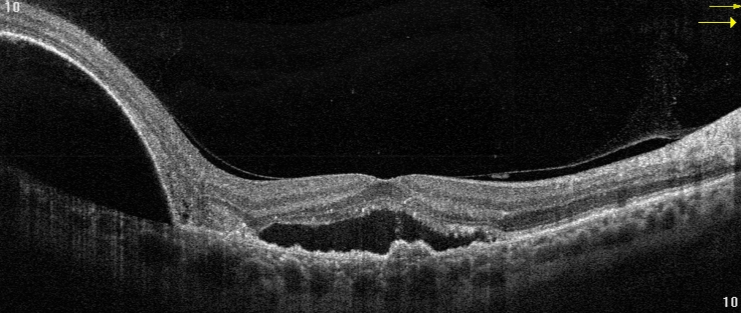
Macular OCT demonstrating age-related macular degeneration.